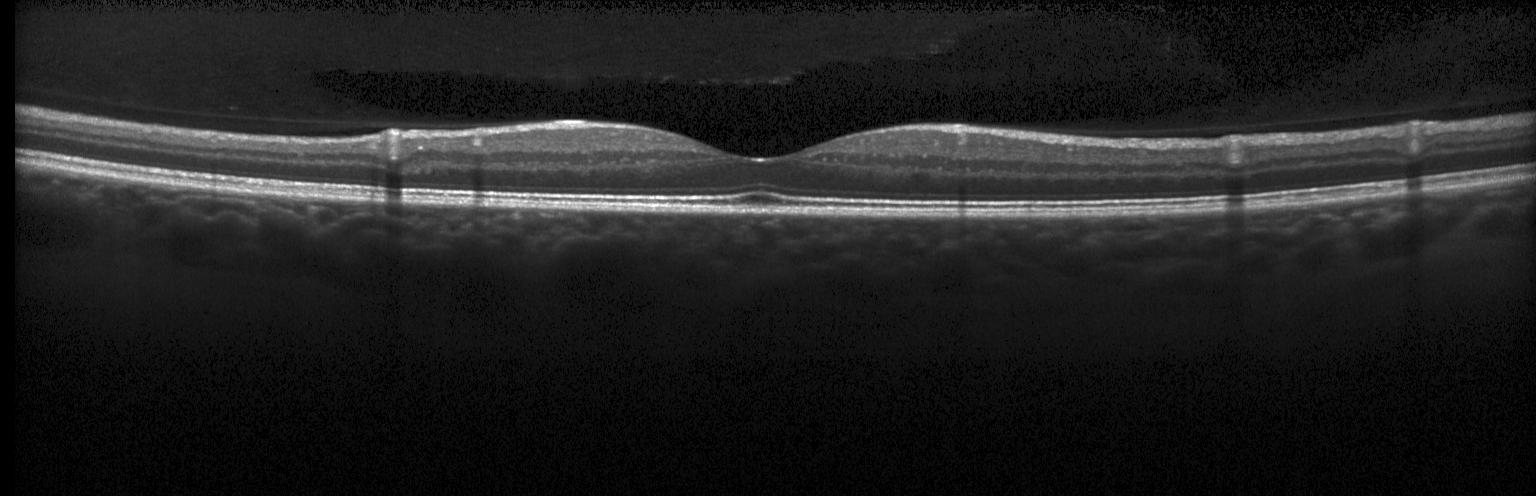
Spectral-domain optical coherence tomography · OCT B-scan · fovea-centered · Heidelberg Spectralis OCT system.
OCT finding: no choroidal neovascularization, no diabetic macular edema, and no drusen.